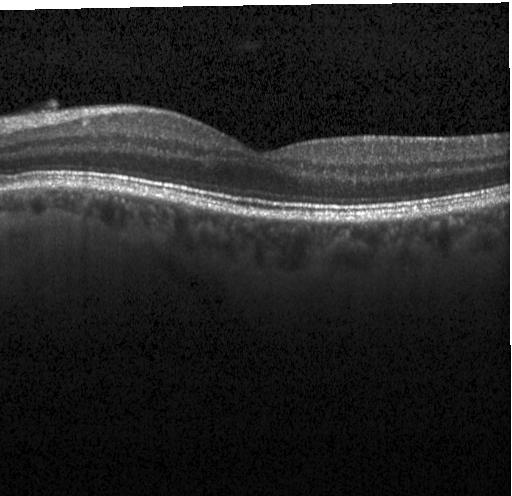 Optical coherence tomography B-scan — Macular OCT: no CNV, no DME, and no drusen.